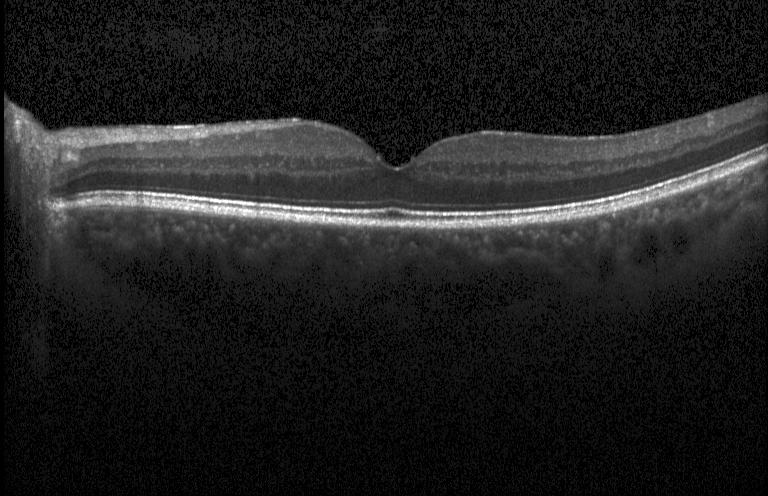

Optical coherence tomography scan — Impression: no CNV, no DME, and no drusen.